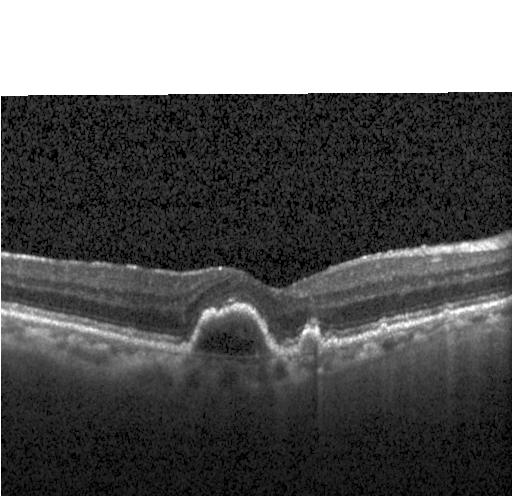 Macular OCT: a choroidal neovascular membrane.